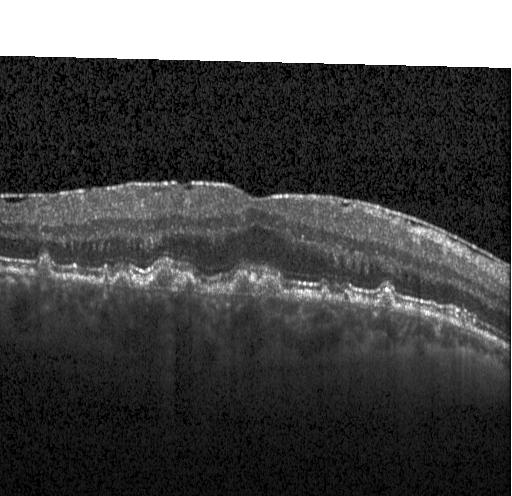
Retinal OCT B-scan. OCT finding: multiple drusen.